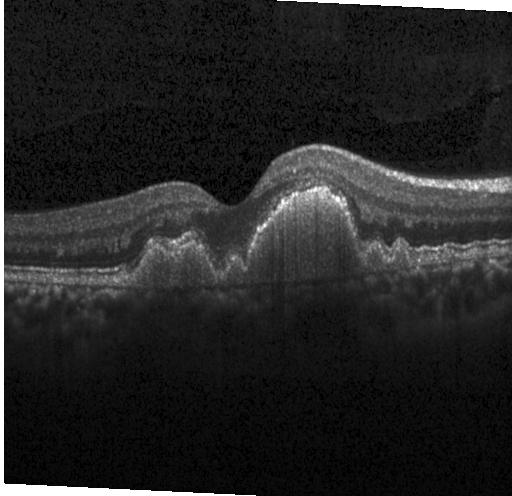 Impression: drusen.